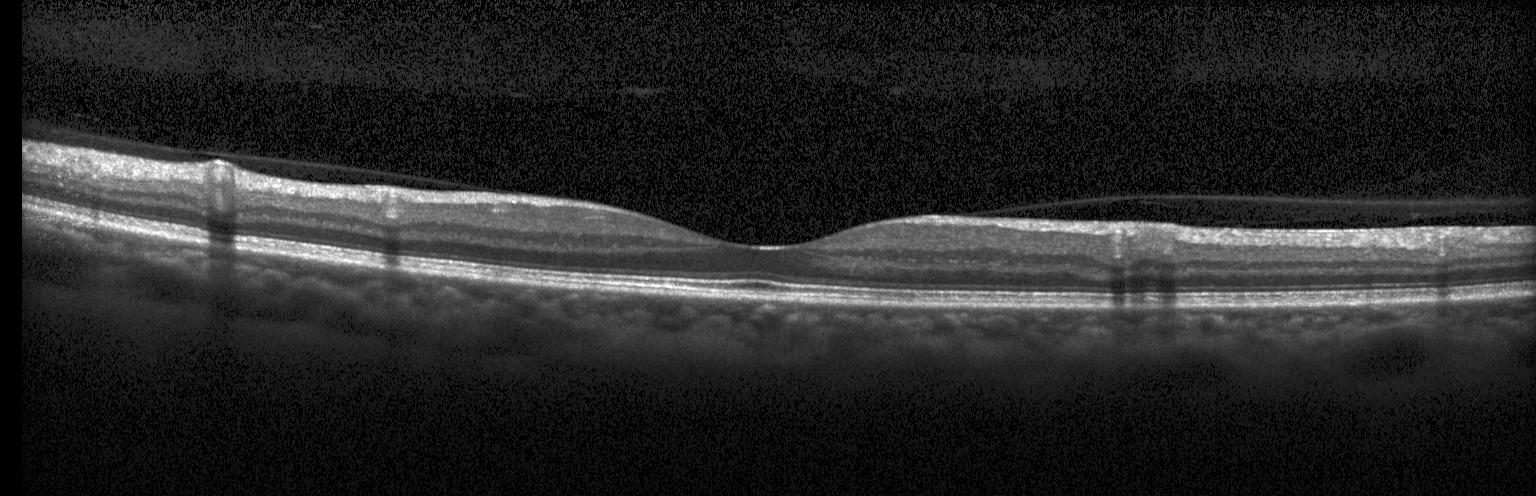
Macular OCT: neither choroidal neovascularization, diabetic macular edema, nor drusen.